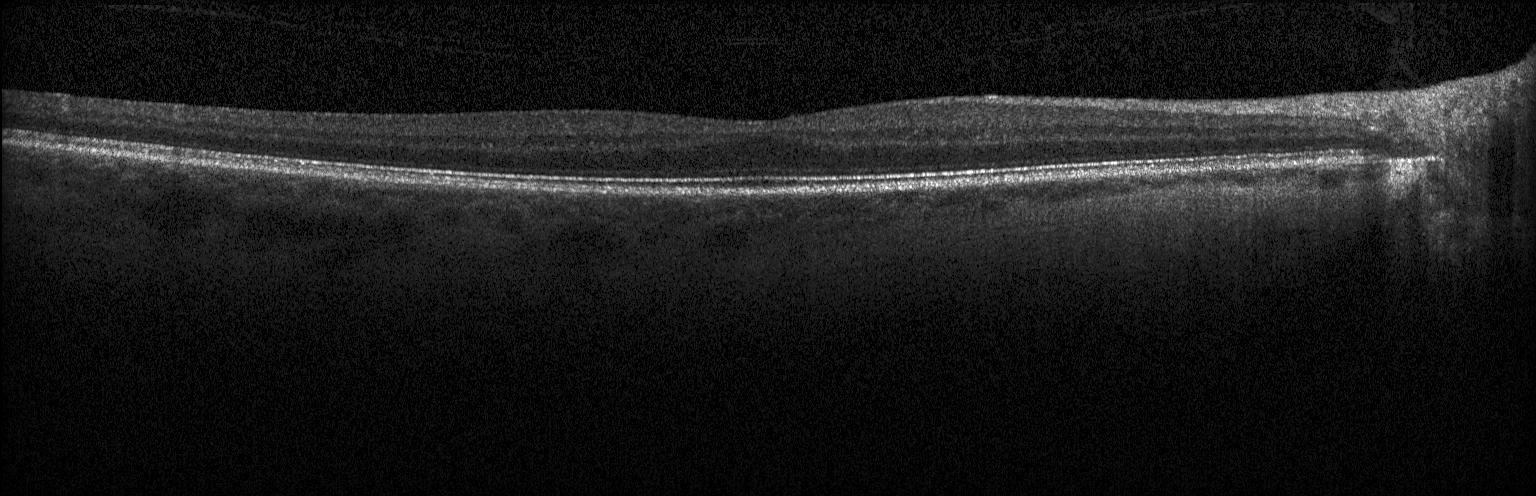

No choroidal neovascularization, no diabetic macular edema, and no drusen.